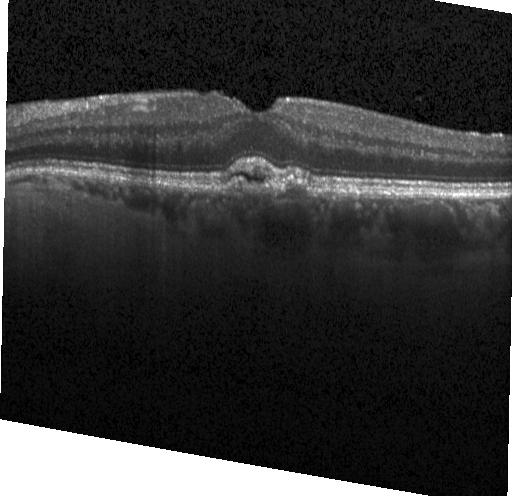

Optical coherence tomography scan · Heidelberg Spectralis.
The scan shows CNV.